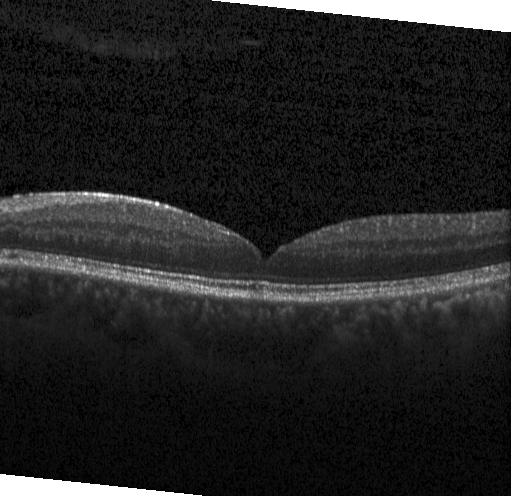
Retinal OCT cross-section — Assessment: no evidence of CNV, DME, or drusen.